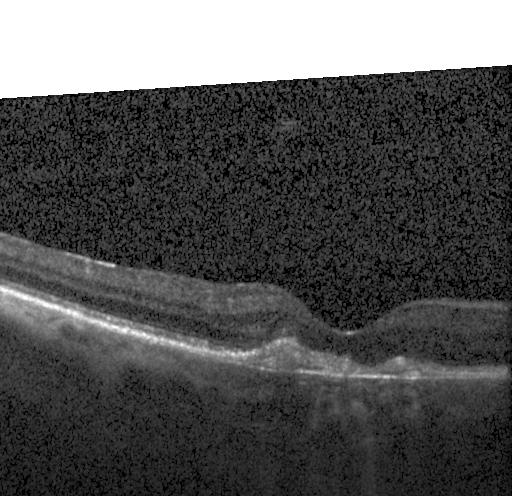

Heidelberg Spectralis OCT system, retinal OCT B-scan
Impression: CNV.